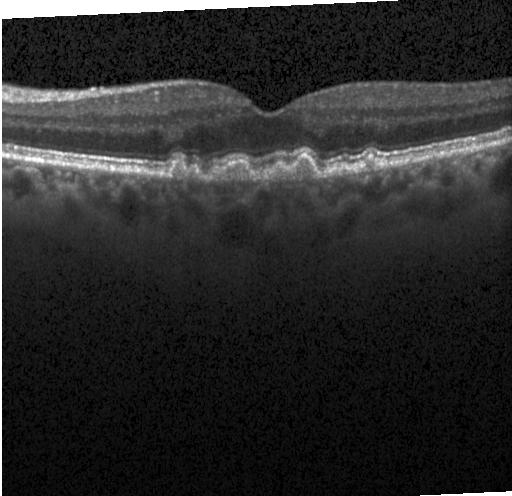 Spectral-domain OCT. Optical coherence tomography B-scan. Horizontal scan through the fovea.
This B-scan demonstrates multiple drusen.